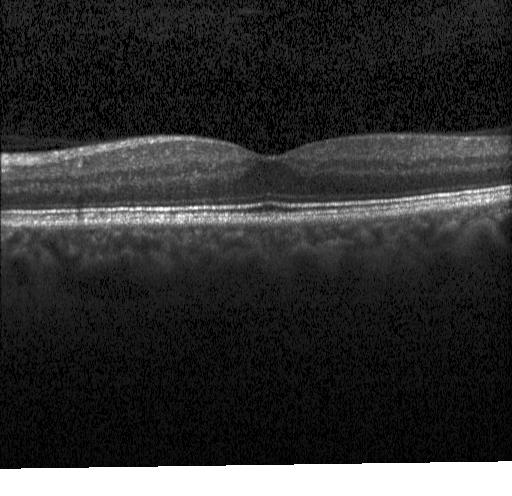 Retinal OCT cross-section. Heidelberg Spectralis OCT system
OCT finding: no choroidal neovascularization, diabetic macular edema, or drusen.